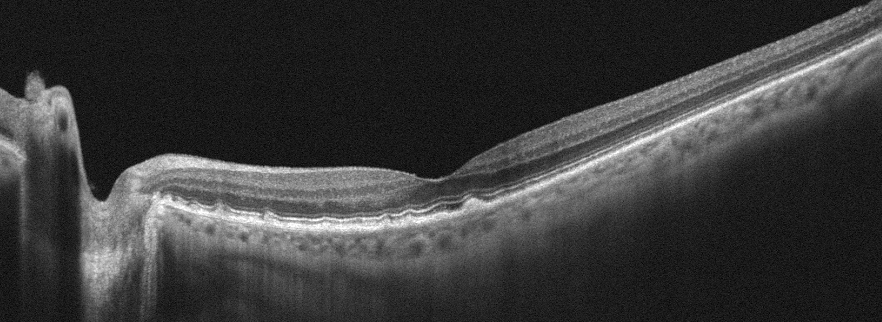

Retinal OCT B-scan. Oculus sinister
Diagnosis: age-related macular degeneration (AMD).